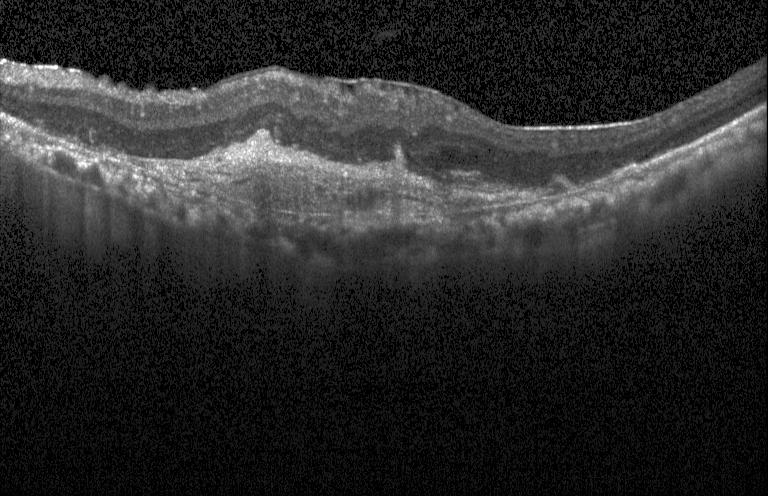
Finding: a choroidal neovascular membrane.